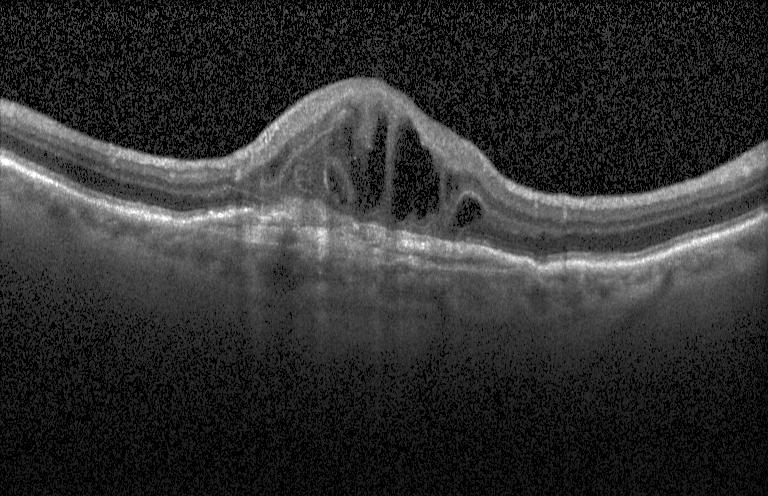
Retinal OCT cross-section.
This B-scan demonstrates CNV.